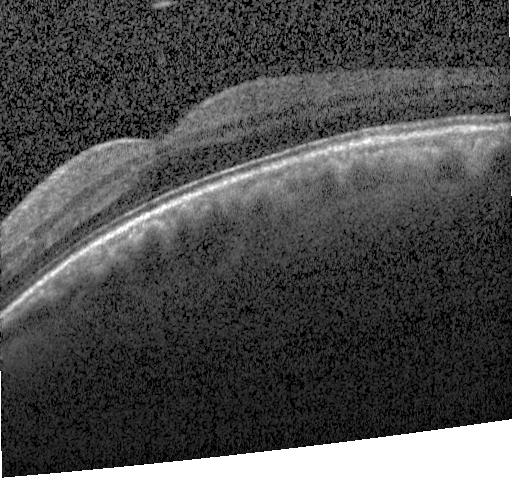

OCT B-scan
Assessment: no evidence of choroidal neovascularization, diabetic macular edema, or drusen.